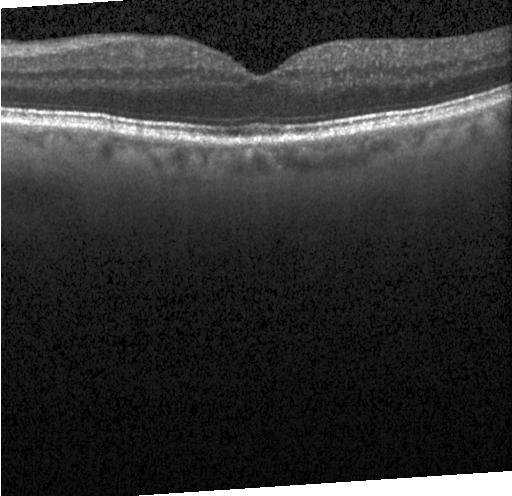 Horizontal scan through the fovea. OCT B-scan.
Diagnosis: neither choroidal neovascularization, diabetic macular edema, nor drusen.